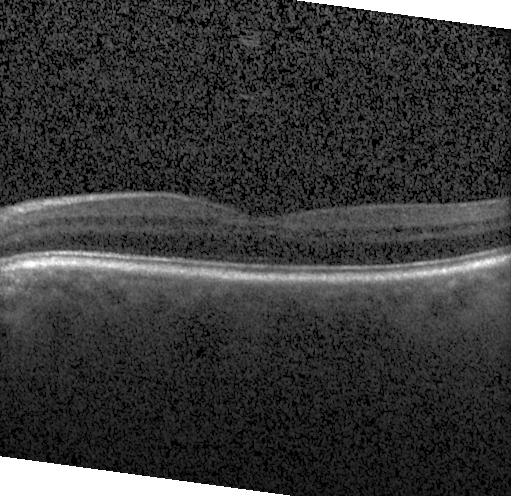

Retinal OCT B-scan; spectral-domain optical coherence tomography; instrument: Heidelberg Spectralis
Finding: neither CNV, DME, nor drusen.